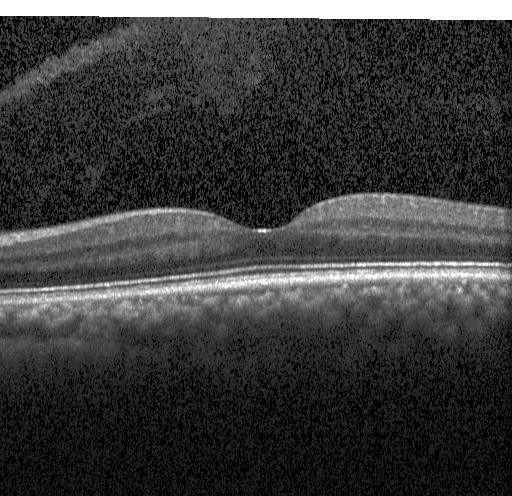 This B-scan demonstrates no choroidal neovascularization, no diabetic macular edema, and no drusen.